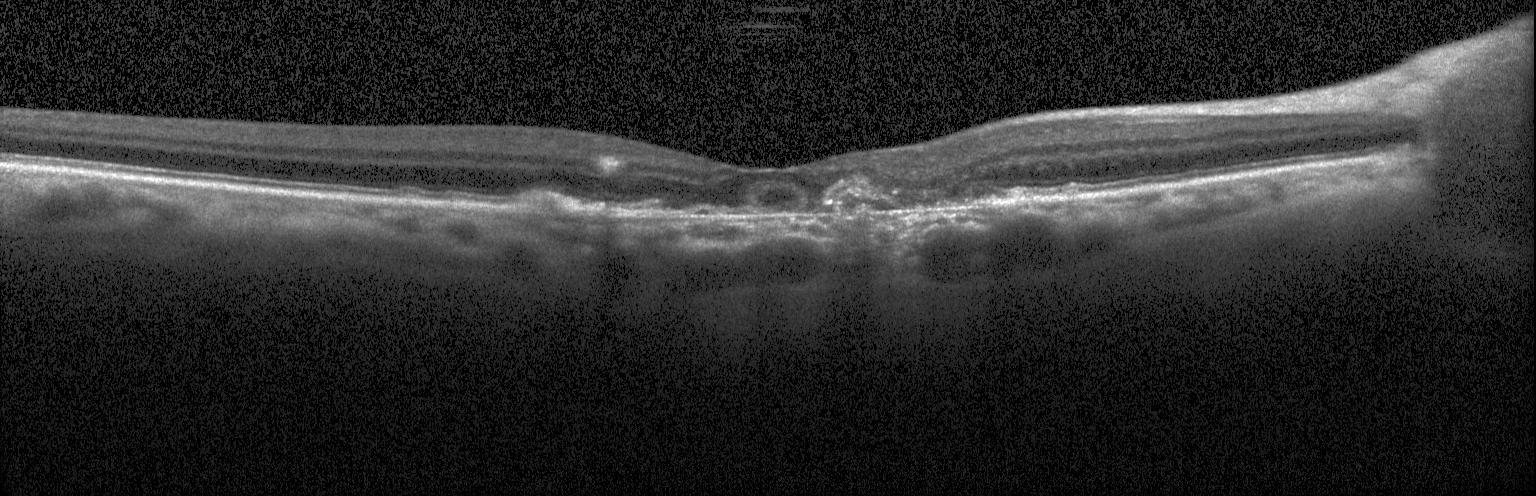
Spectral-domain OCT B-scan: choroidal neovascularization.